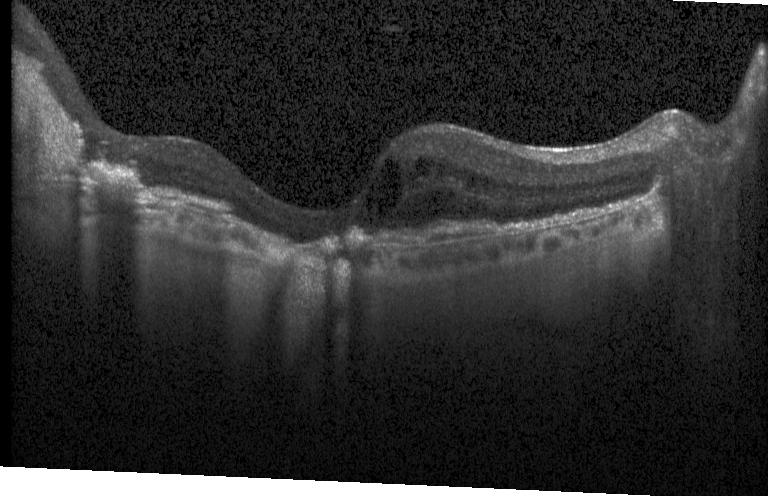

Impression: choroidal neovascularization.